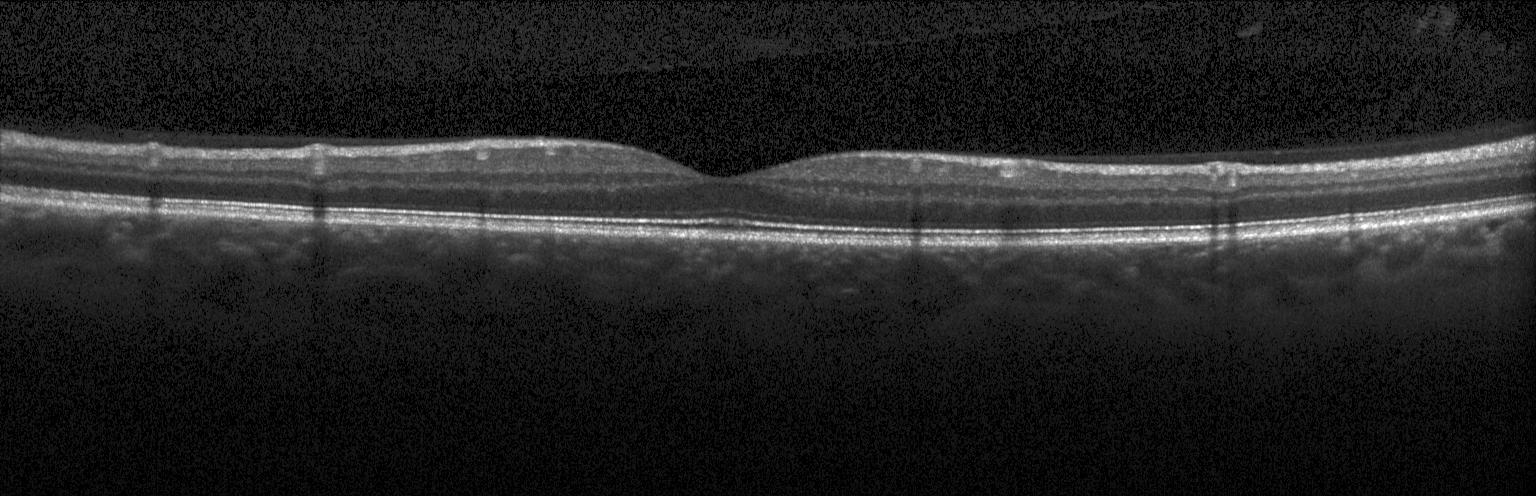

Finding: no choroidal neovascularization, diabetic macular edema, or drusen.